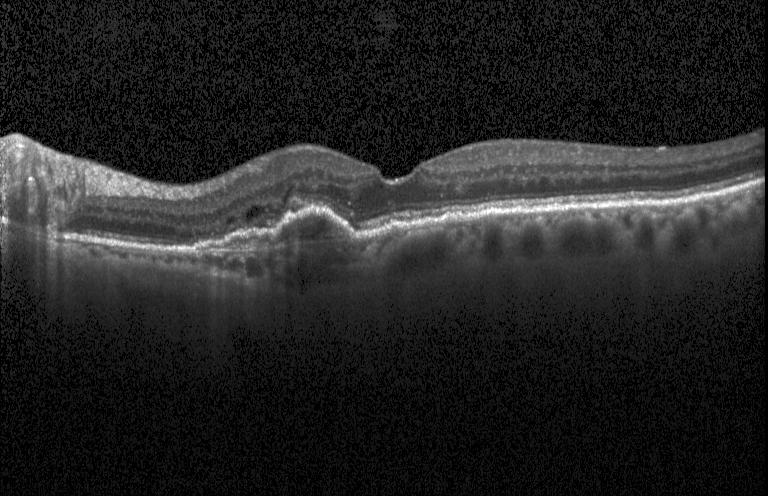

Retinal OCT B-scan. Horizontal scan through the fovea. Heidelberg Spectralis.
Macular OCT: CNV.